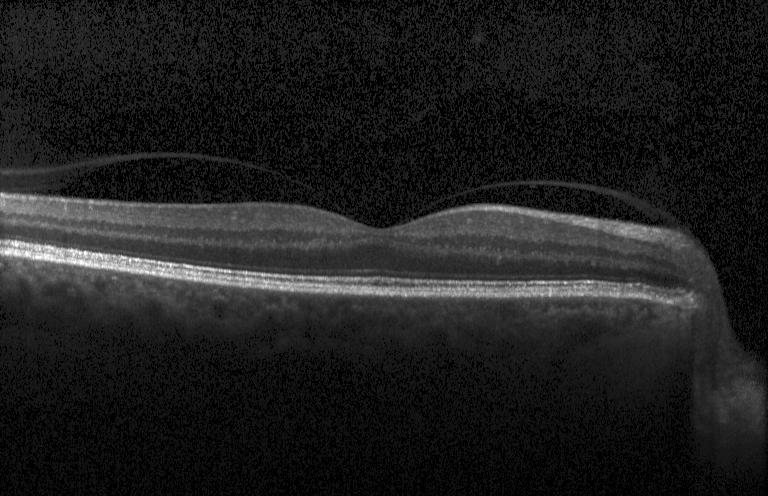 OCT line scan.
Impression: no evidence of choroidal neovascularization, diabetic macular edema, or drusen.